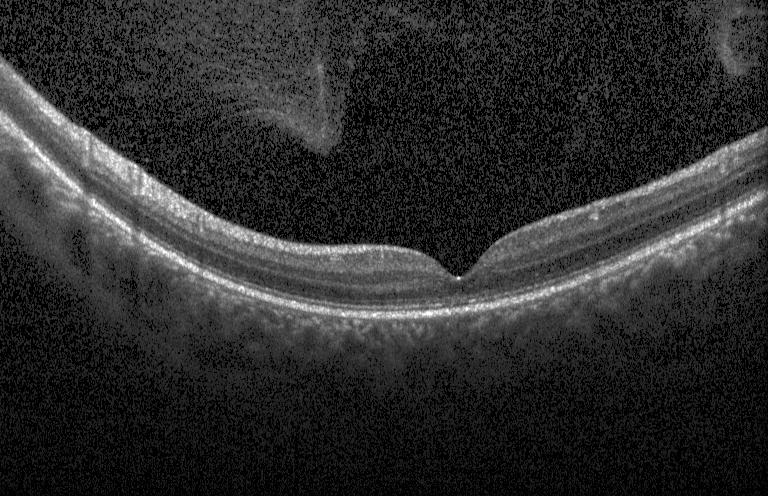 Finding: no choroidal neovascularization, diabetic macular edema, or drusen.